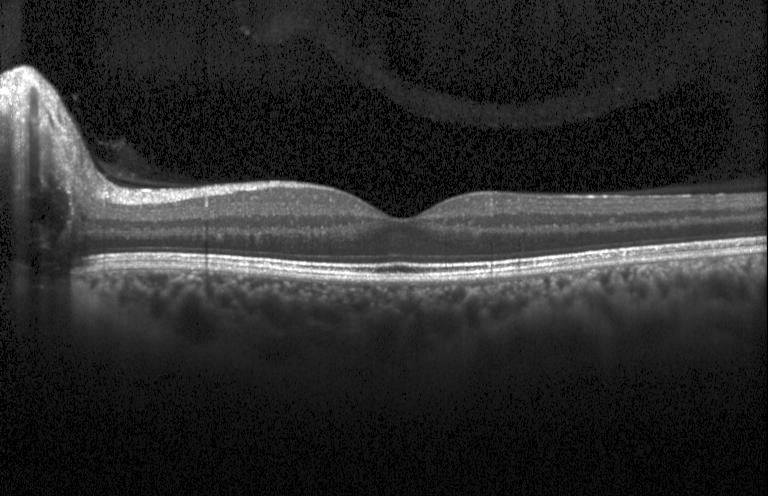

SD-OCT, OCT B-scan
OCT finding: neither choroidal neovascularization, diabetic macular edema, nor drusen.